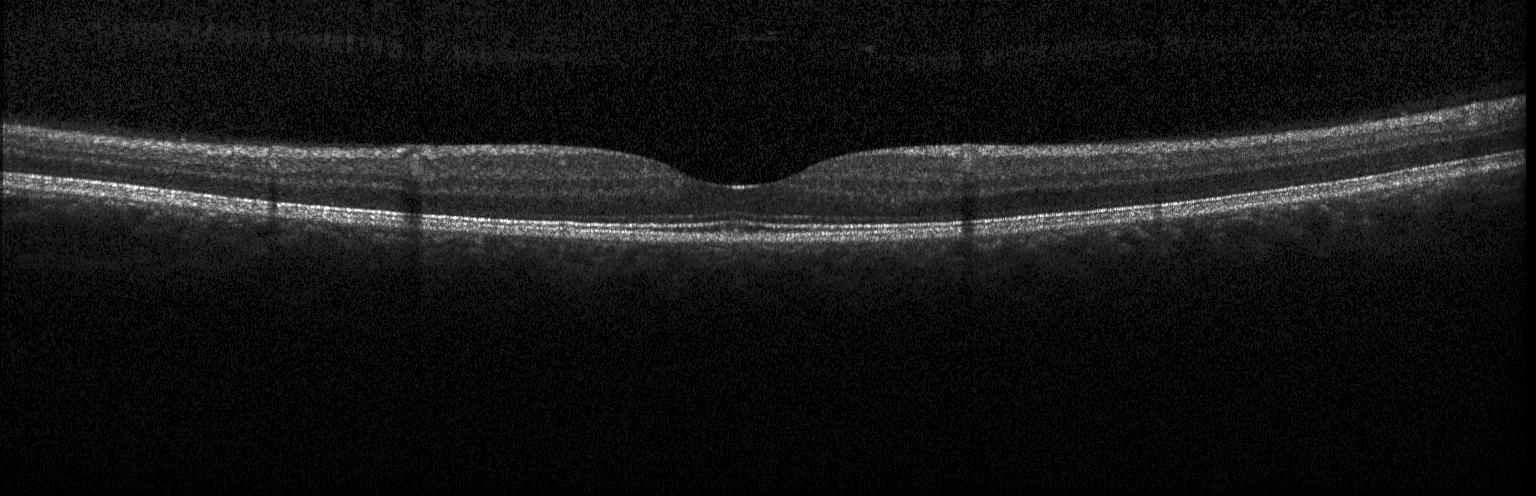
OCT B-scan showing no evidence of choroidal neovascularization, diabetic macular edema, or drusen.